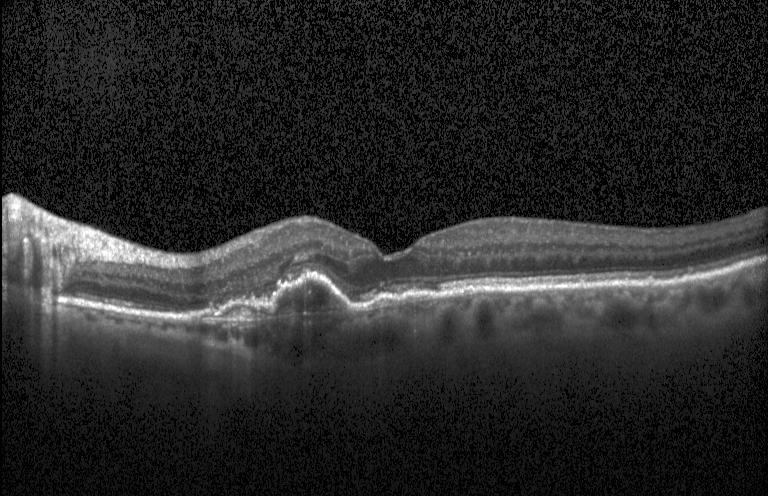

Heidelberg Spectralis, retinal OCT cross-section. A choroidal neovascular membrane.